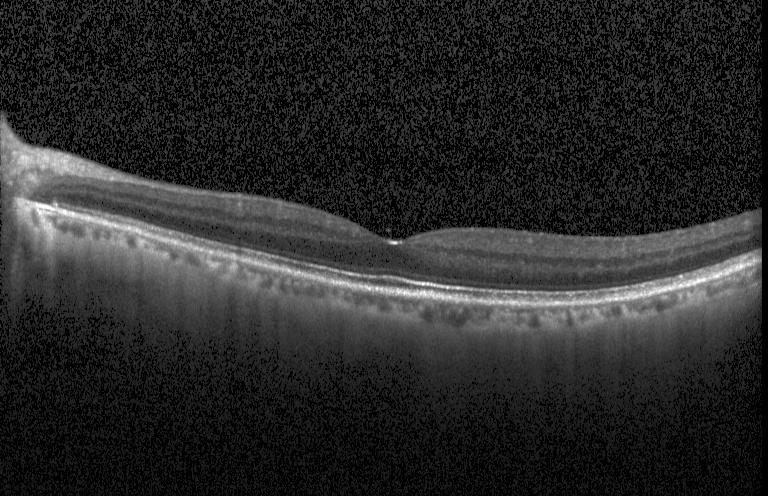

Optical coherence tomography scan, macular scan, SD-OCT — Impression: no evidence of choroidal neovascularization, diabetic macular edema, or drusen.